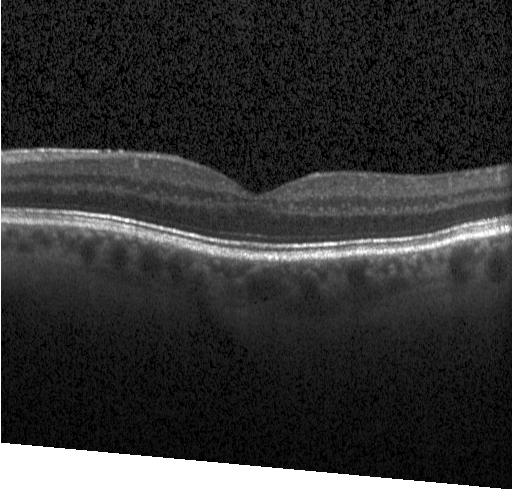

OCT finding: no CNV, no DME, and no drusen.